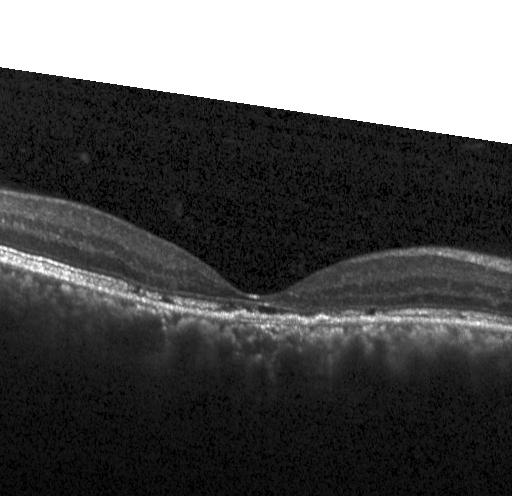

Impression: a choroidal neovascular membrane.